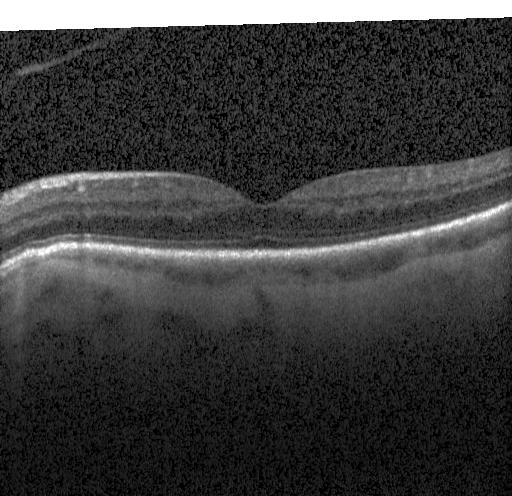
Finding: no CNV, no DME, and no drusen.